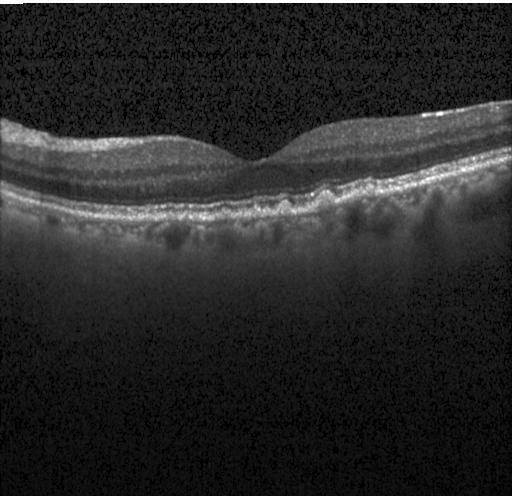 SD-OCT · retinal OCT B-scan.
Finding: drusen.